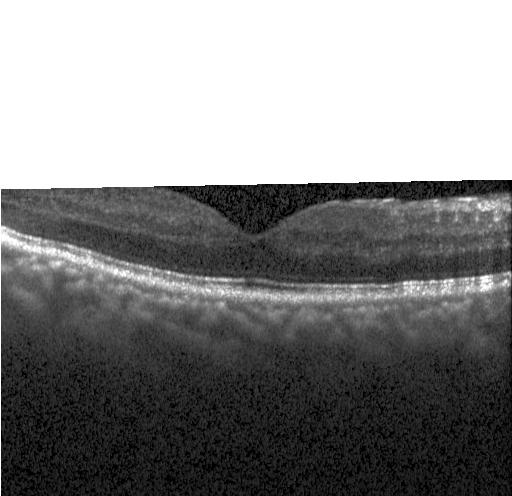 Through the macula. Spectral-domain OCT. Optical coherence tomography B-scan. Acquired on a Heidelberg Spectralis
Macular OCT: neither choroidal neovascularization, diabetic macular edema, nor drusen.